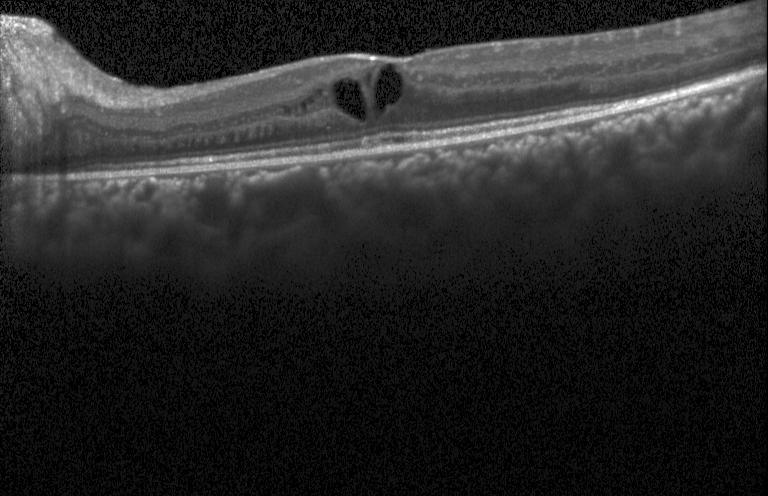

SD-OCT; optical coherence tomography scan. Assessment: diabetic macular edema (DME).